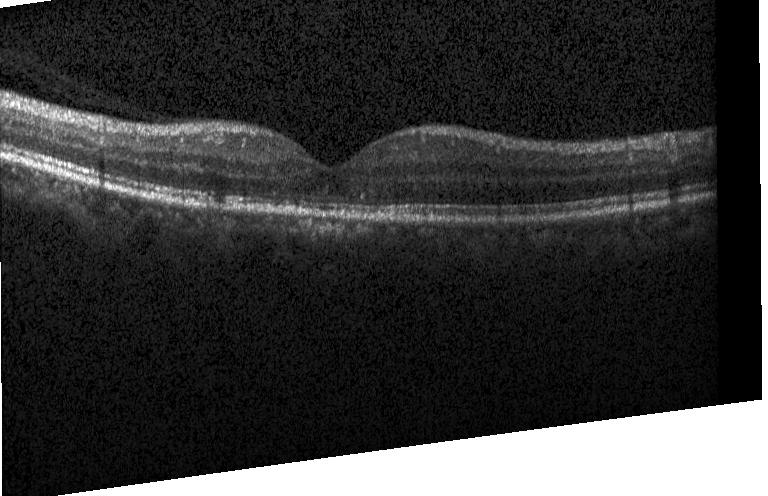

Macular scan, optical coherence tomography B-scan.
Diagnosis: no choroidal neovascularization, diabetic macular edema, or drusen.